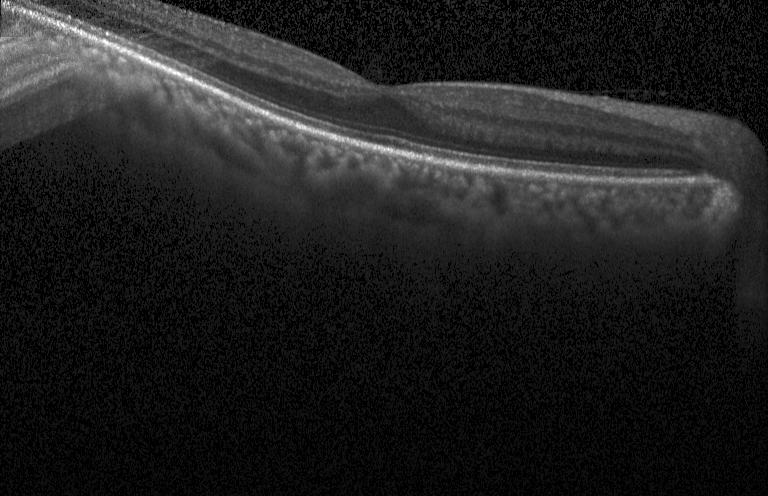 Finding: no choroidal neovascularization, no diabetic macular edema, and no drusen.